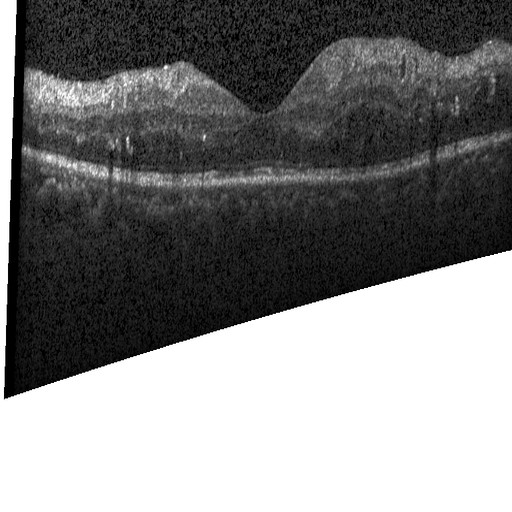

OCT finding: diabetic macular edema.